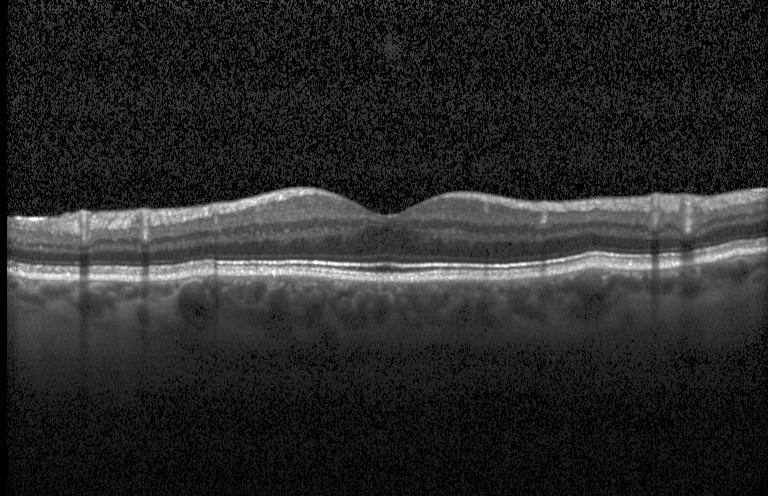

Finding: neither choroidal neovascularization, diabetic macular edema, nor drusen.